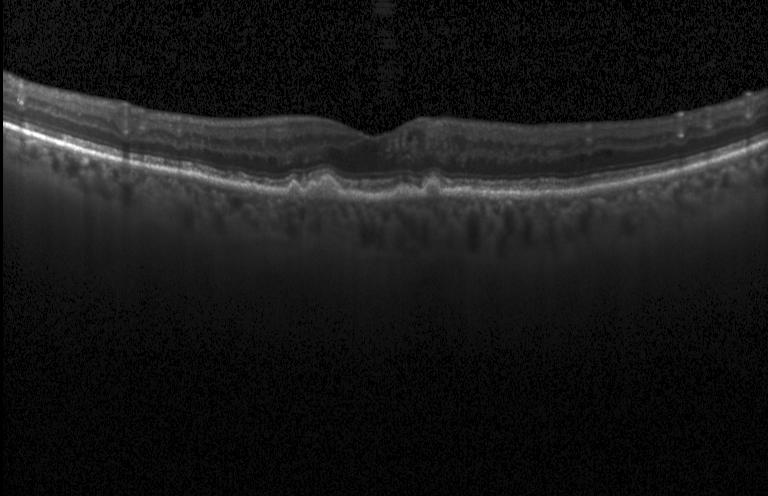
Finding: multiple drusen.